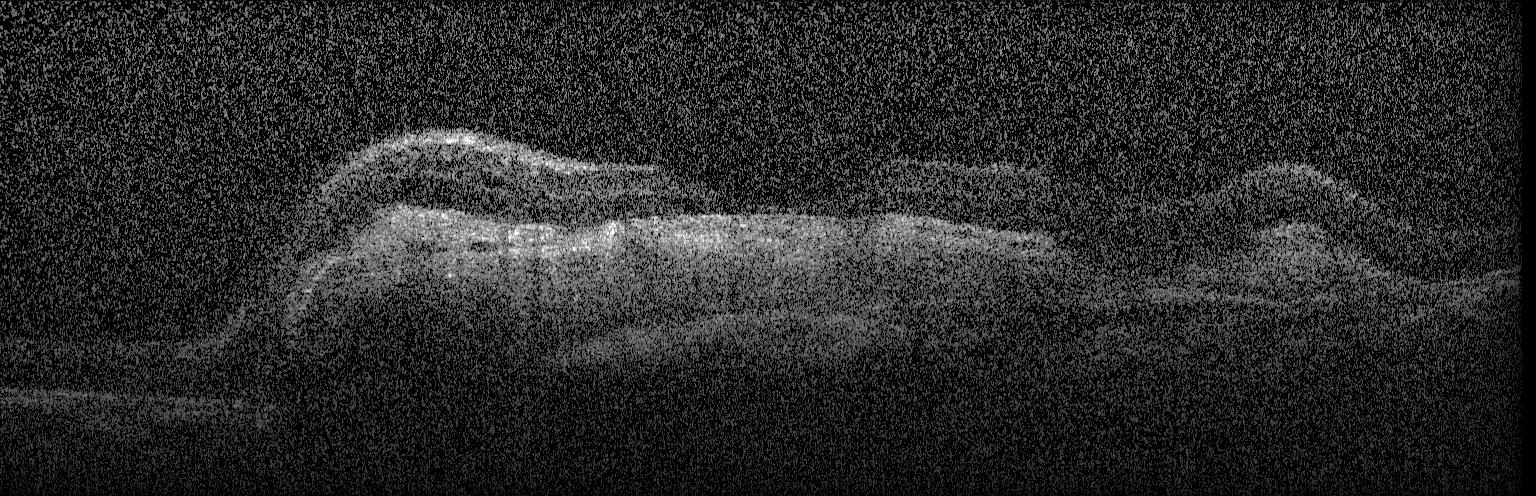 Optical coherence tomography scan — Diagnosis: a choroidal neovascular membrane.